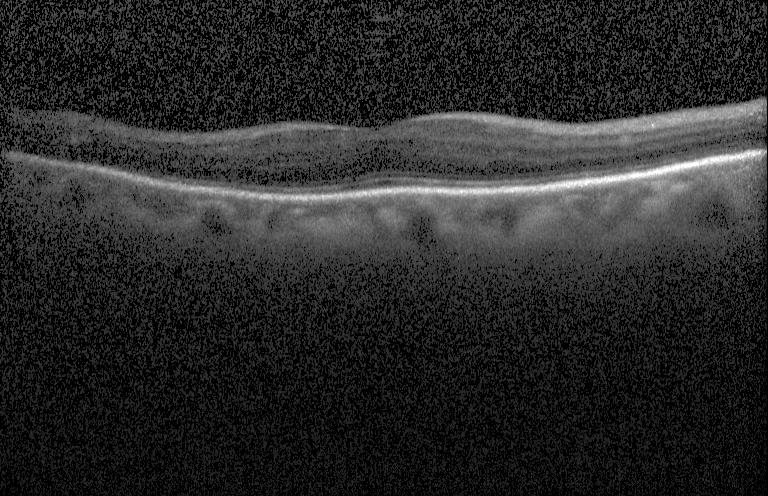
Fovea-centered · spectral-domain OCT · OCT B-scan
The scan shows no evidence of choroidal neovascularization, diabetic macular edema, or drusen.